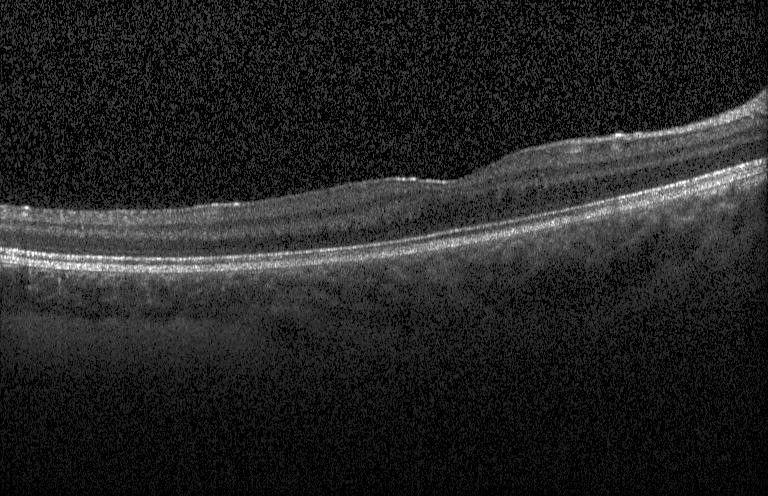 Optical coherence tomography B-scan
Macular OCT: neither choroidal neovascularization, diabetic macular edema, nor drusen.